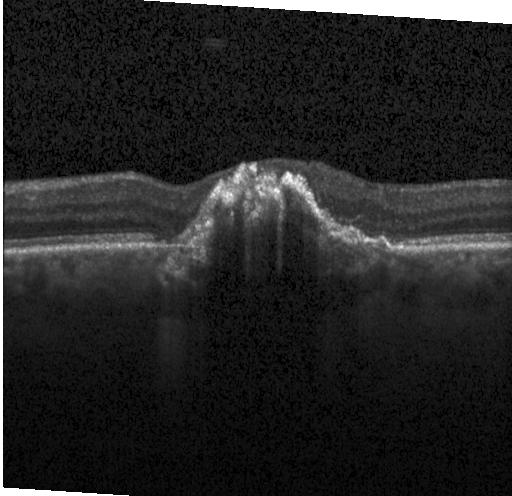
Retinal OCT B-scan. Spectral-domain OCT
Diagnosis: a choroidal neovascular membrane.